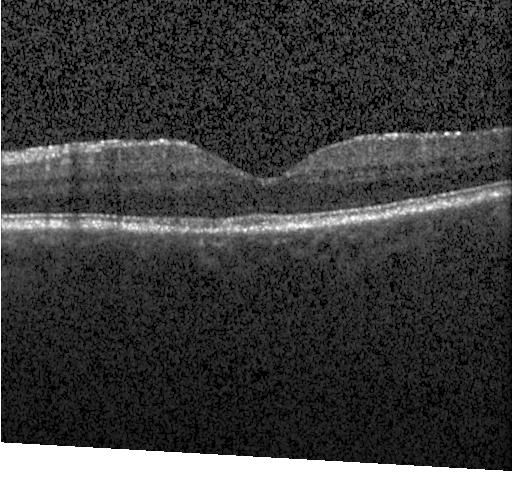 Impression: neither choroidal neovascularization, diabetic macular edema, nor drusen.